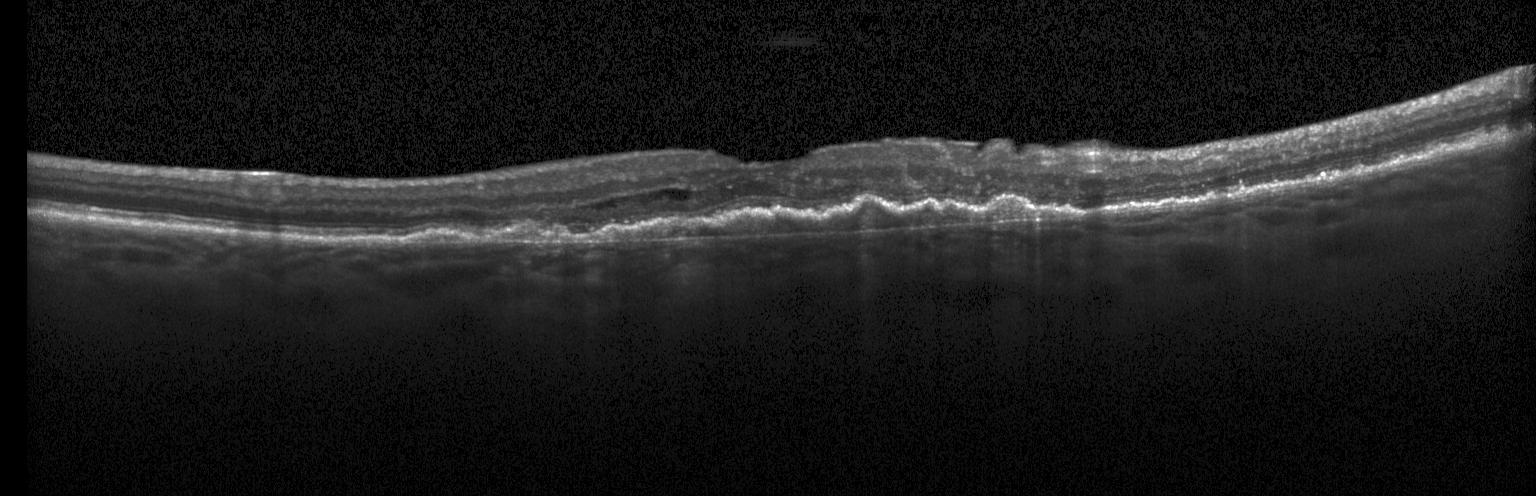

The scan shows a choroidal neovascular membrane.